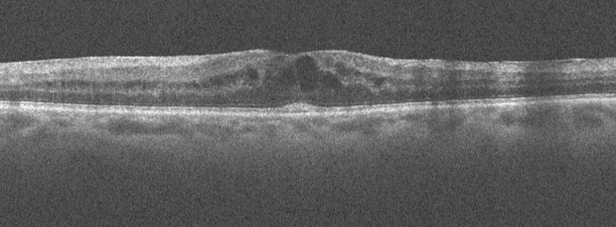

Optical coherence tomography B-scan; macular scan; instrument: Optovue Avanti RTVue XR.
Diagnosis: DME.